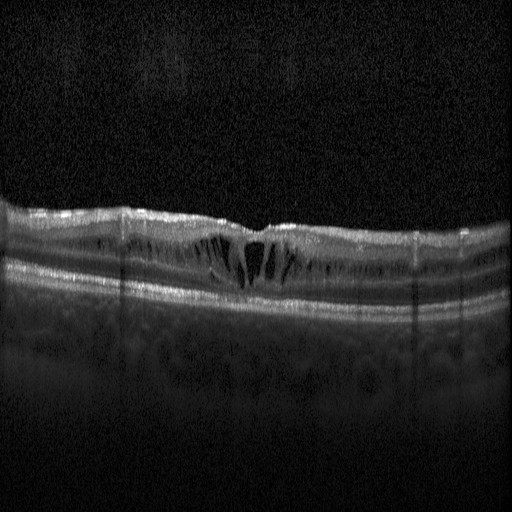
OCT line scan; macular scan. Dx: DME.